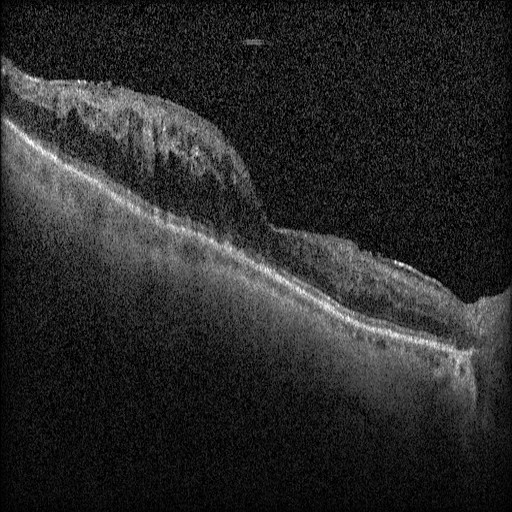

Retinal OCT cross-section; spectral-domain OCT
Impression: DME.